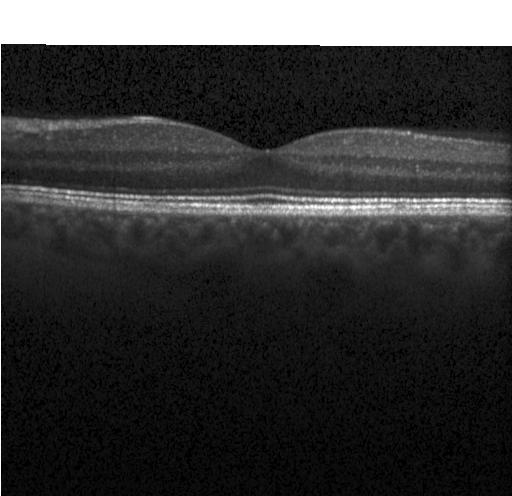

Heidelberg Spectralis, OCT B-scan, spectral-domain optical coherence tomography. The scan shows no choroidal neovascularization, no diabetic macular edema, and no drusen.